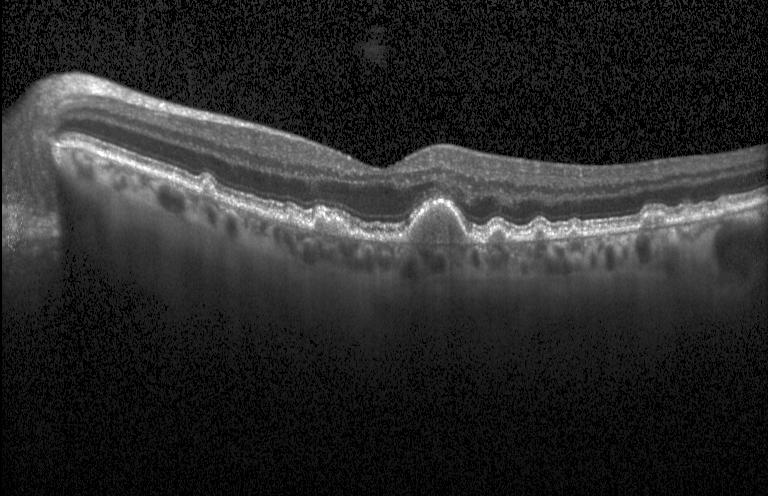 Optical coherence tomography scan, through the macula.
Dx: drusen.